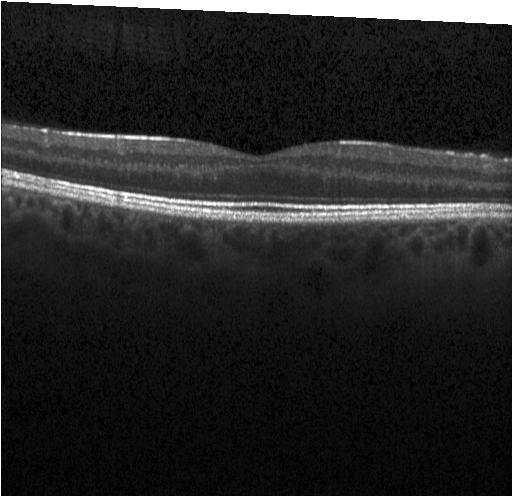
Retinal OCT cross-section, horizontal scan through the fovea, Heidelberg Spectralis
The scan shows no CNV, DME, or drusen.